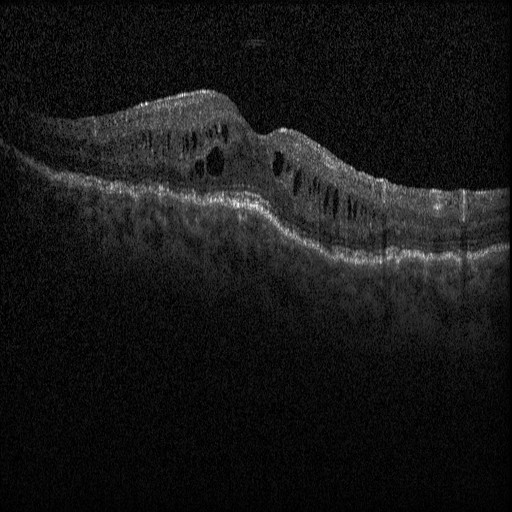

This B-scan demonstrates DME.